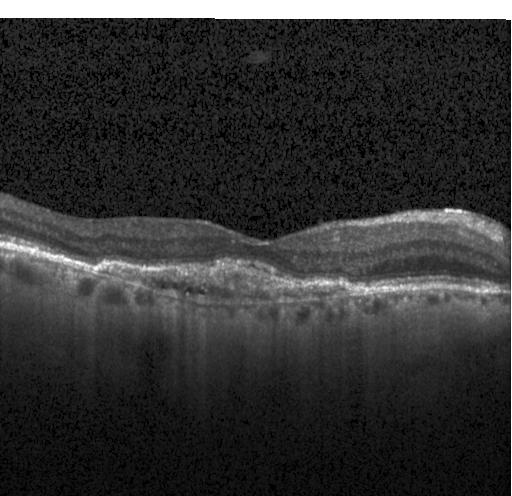
The scan shows CNV.